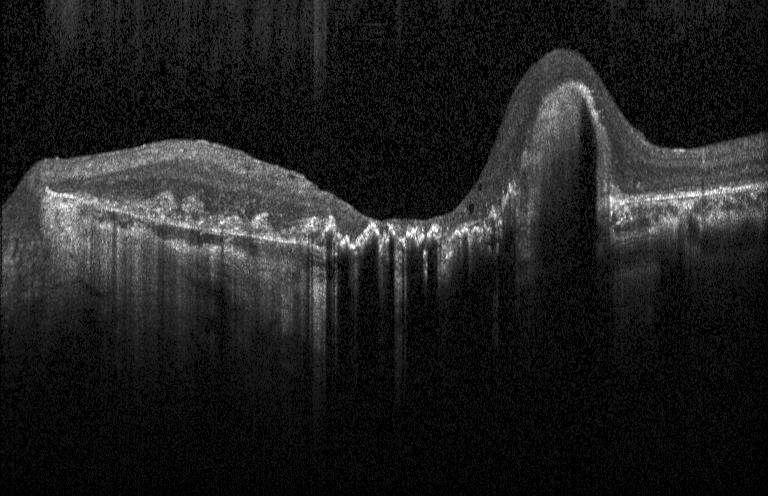
This B-scan demonstrates choroidal neovascularization.